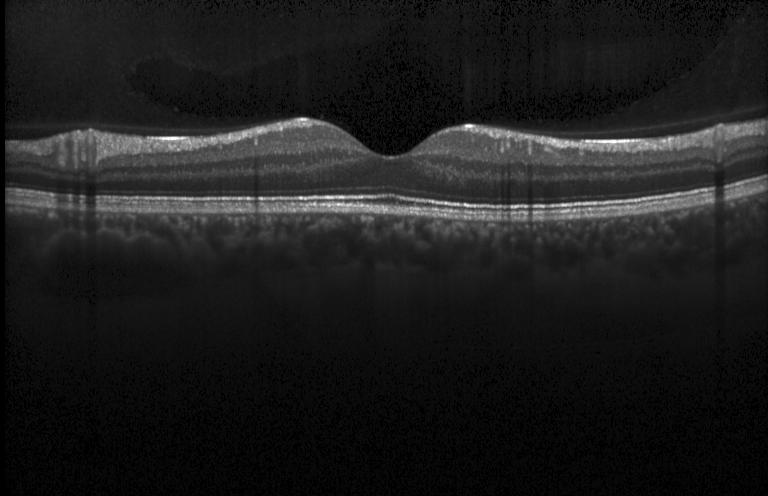

Retinal OCT cross-section, Heidelberg Spectralis, fovea-centered. Macular OCT: no evidence of choroidal neovascularization, diabetic macular edema, or drusen.